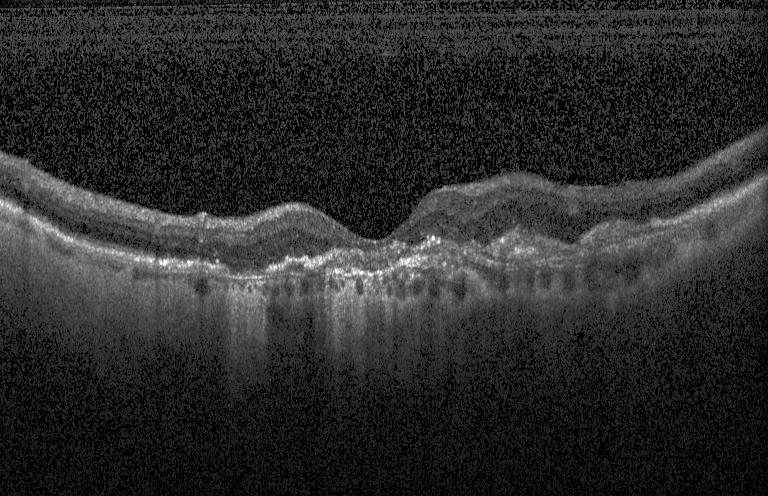 Finding: a choroidal neovascular membrane.